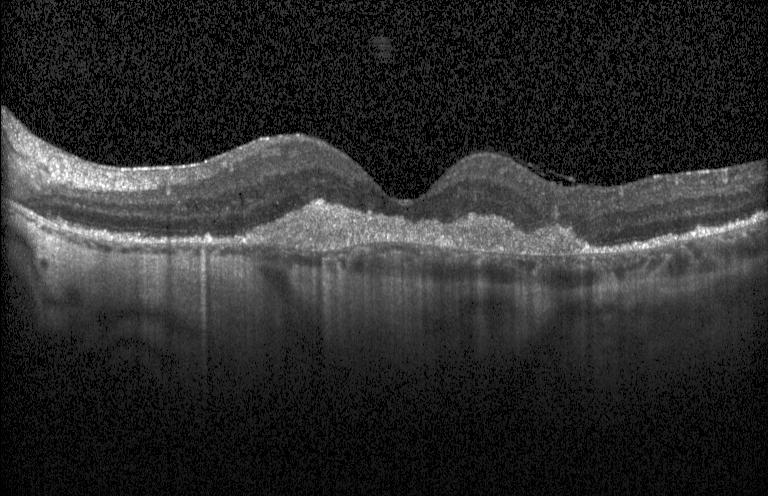
Instrument: Heidelberg Spectralis; retinal OCT cross-section; SD-OCT; fovea-centered.
Finding: a choroidal neovascular membrane.